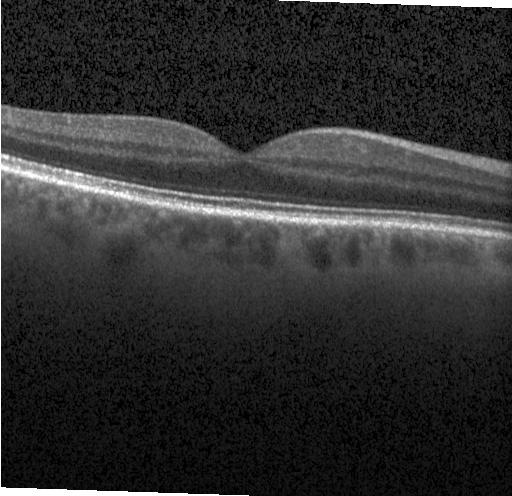
Impression: no CNV, no DME, and no drusen.